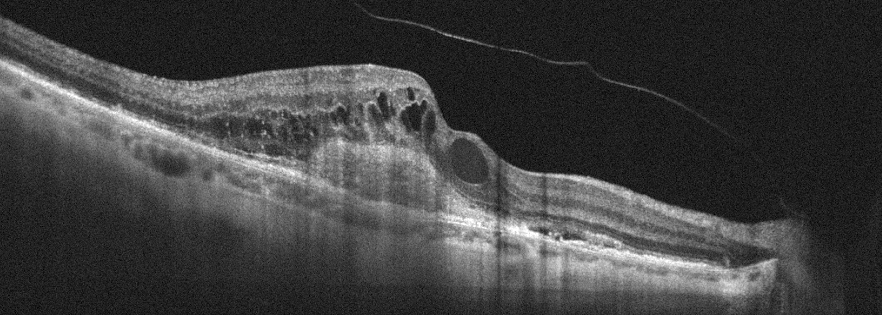 OCT B-scan showing AMD.